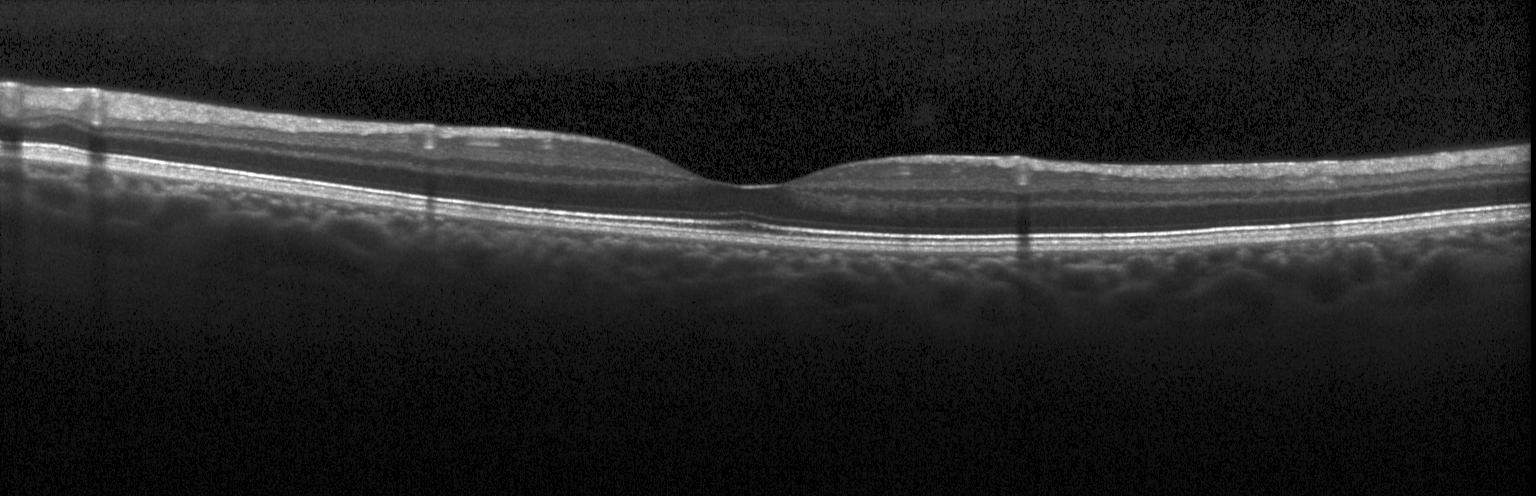

The scan shows no choroidal neovascularization, no diabetic macular edema, and no drusen.